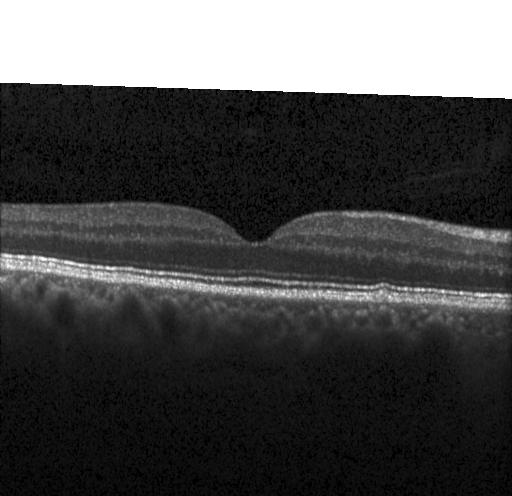

Fovea-centered · retinal OCT cross-section · acquired on a Heidelberg Spectralis · SD-OCT. Diagnosis: no evidence of choroidal neovascularization, diabetic macular edema, or drusen.